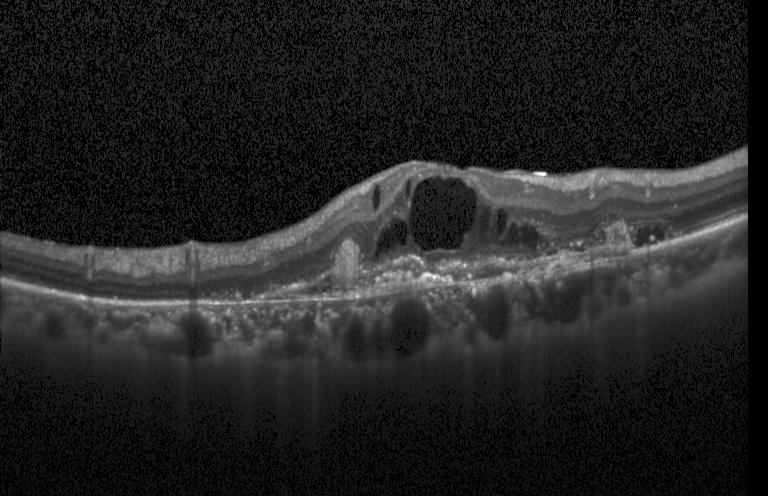 OCT B-scan, spectral-domain OCT — Impression: a choroidal neovascular membrane.